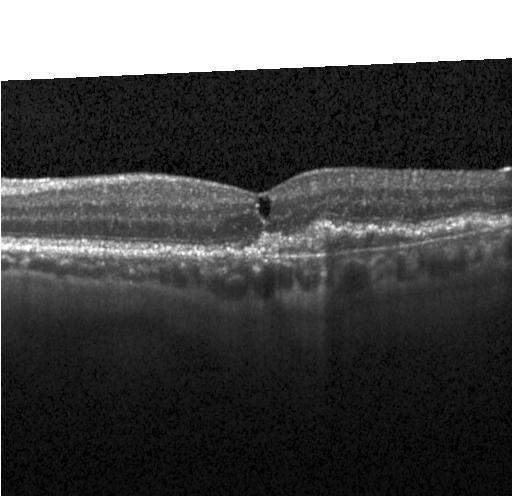 Horizontal scan through the fovea · retinal OCT B-scan. OCT finding: choroidal neovascularization.